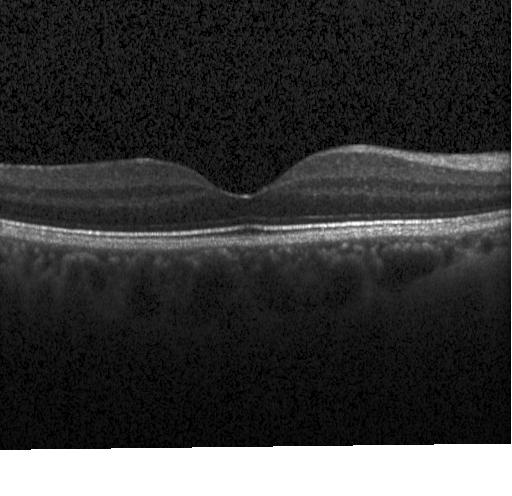 Impression: no CNV, DME, or drusen.